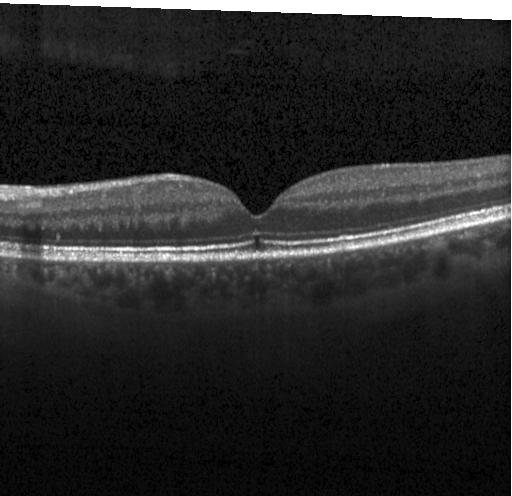

Finding: no choroidal neovascularization, diabetic macular edema, or drusen.